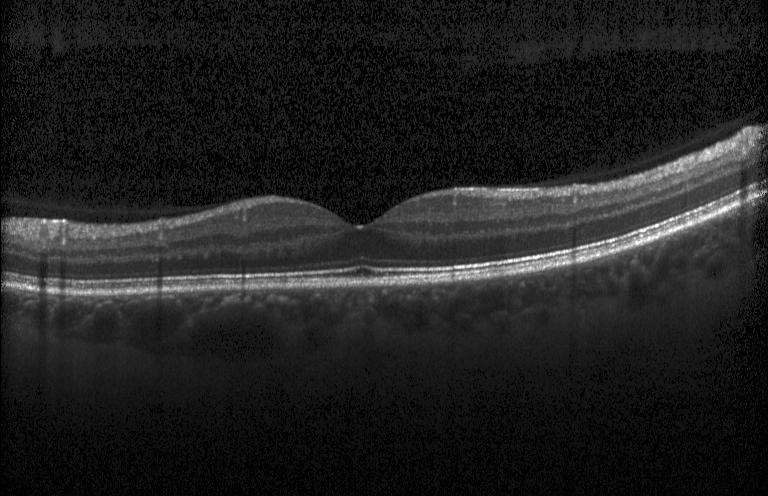

Spectral-domain OCT, OCT B-scan, centered on the fovea
The scan shows no CNV, no DME, and no drusen.